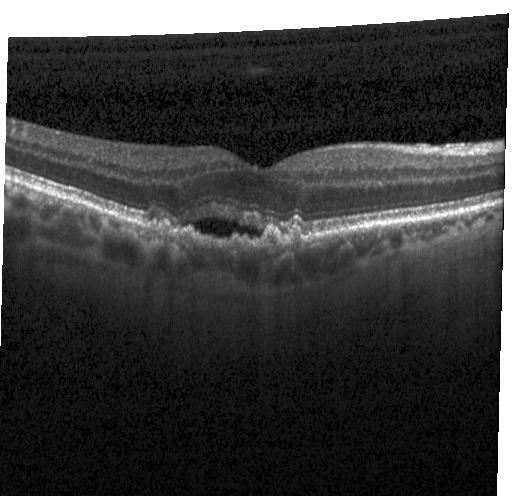

CNV.